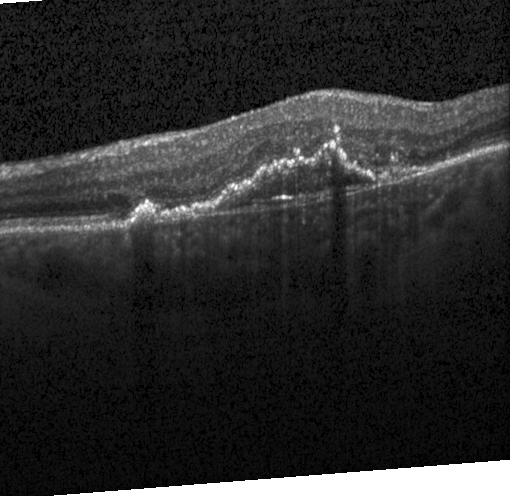
OCT line scan
The scan shows a choroidal neovascular membrane.